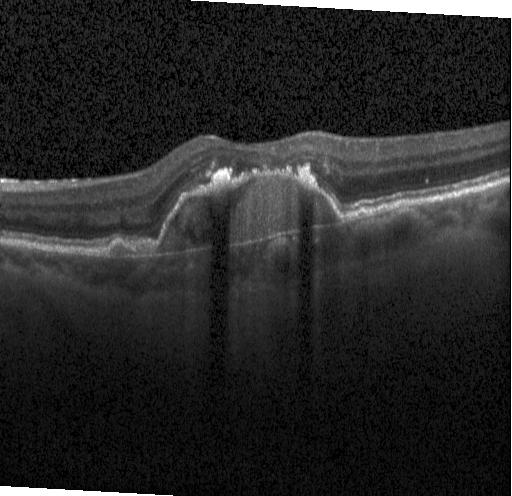

Diagnosis: CNV.